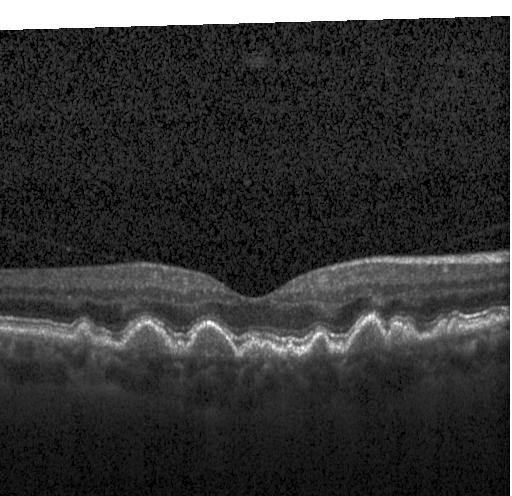
OCT finding: multiple drusen.